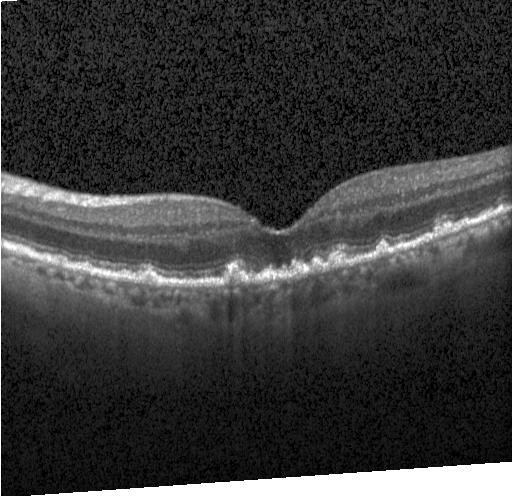

Assessment: sub-RPE drusenoid deposits.